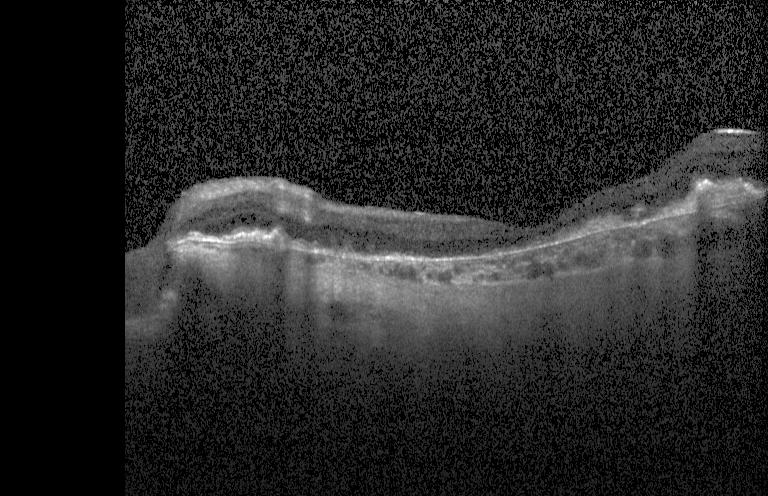
Retinal OCT cross-section showing choroidal neovascularization.